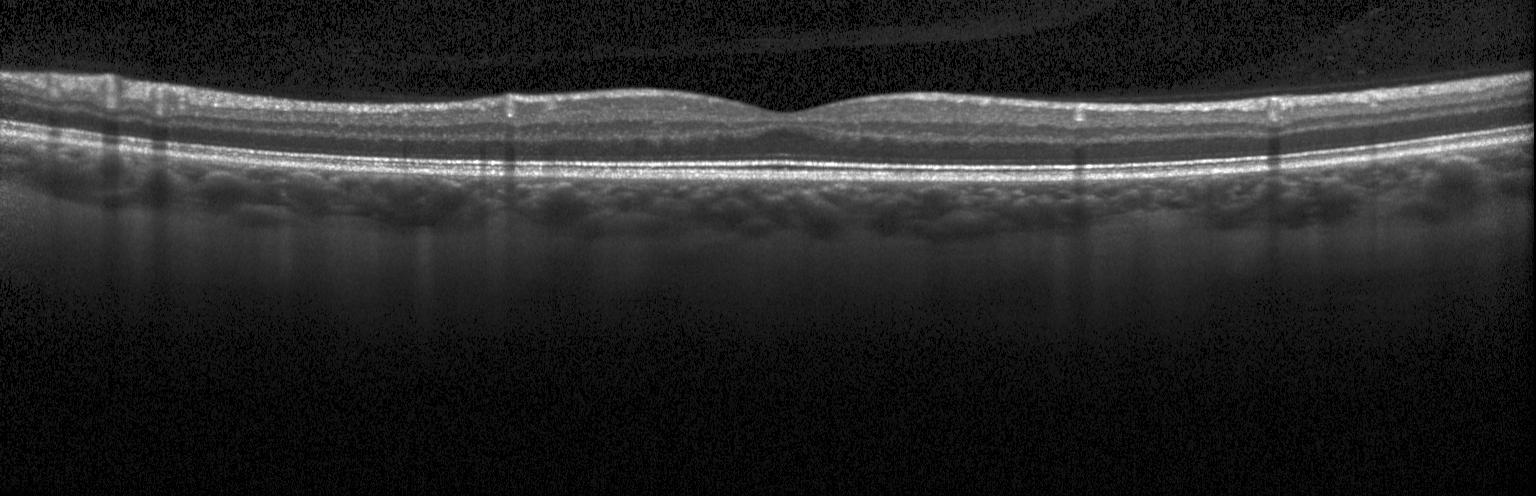

Dx: no choroidal neovascularization, diabetic macular edema, or drusen.